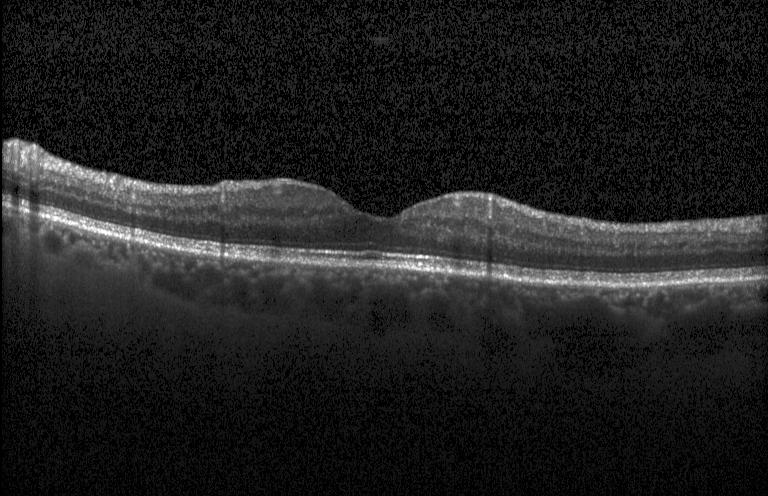

OCT B-scan — Impression: no choroidal neovascularization, diabetic macular edema, or drusen.